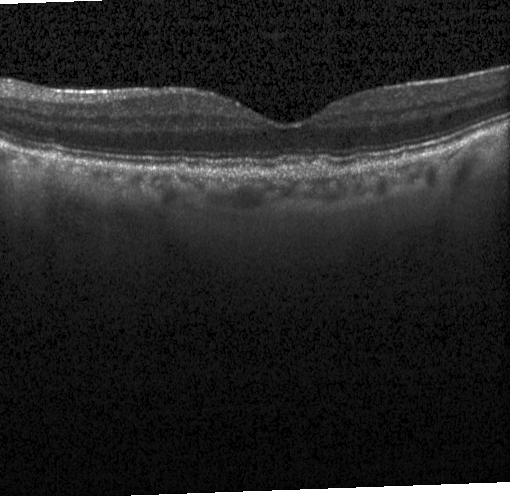

Assessment: multiple drusen.